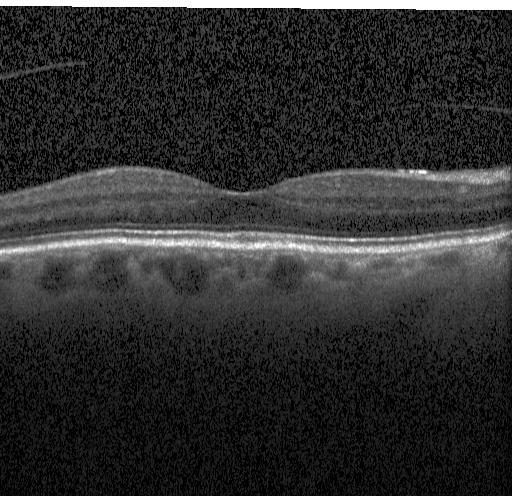
Optical coherence tomography scan, instrument: Heidelberg Spectralis — Diagnosis: no choroidal neovascularization, no diabetic macular edema, and no drusen.